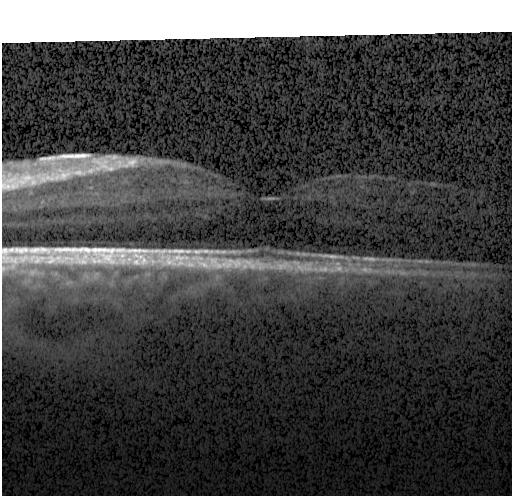 Spectral-domain OCT B-scan: no choroidal neovascularization, diabetic macular edema, or drusen.